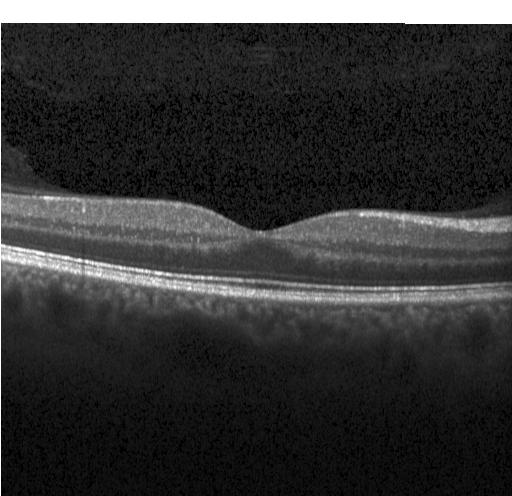 Retinal OCT cross-section.
This B-scan demonstrates no evidence of choroidal neovascularization, diabetic macular edema, or drusen.